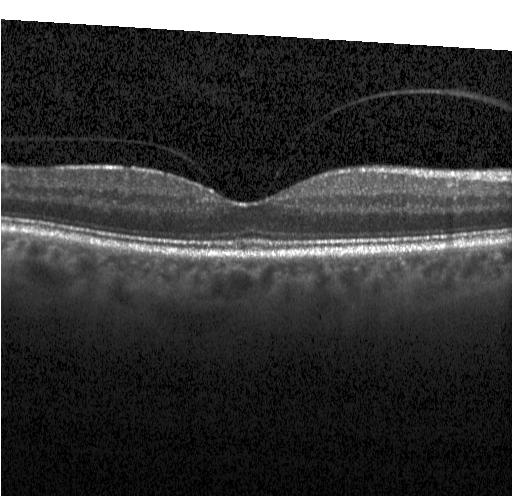
OCT line scan · spectral-domain optical coherence tomography · acquired on a Heidelberg Spectralis — Assessment: no CNV, DME, or drusen.